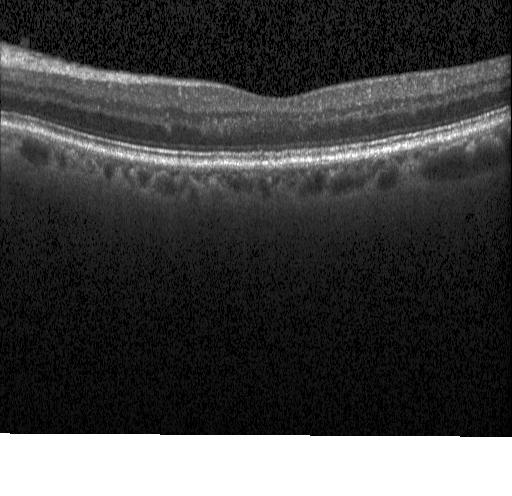
Retinal OCT B-scan; spectral-domain optical coherence tomography. The scan shows no evidence of CNV, DME, or drusen.